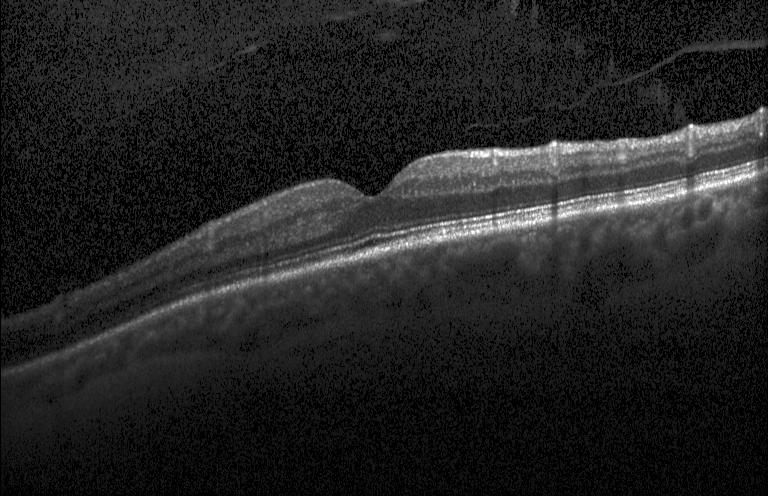

Diagnosis: neither choroidal neovascularization, diabetic macular edema, nor drusen.